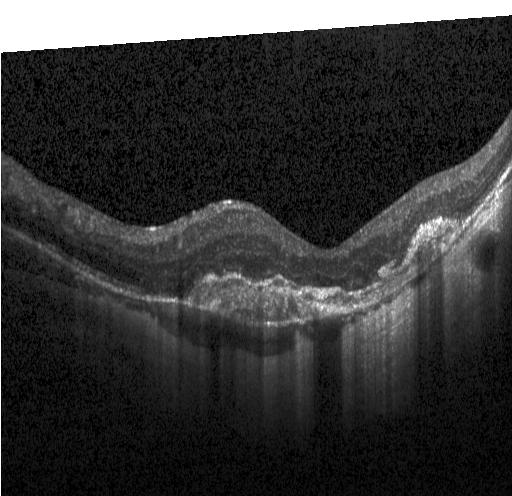
SD-OCT · Heidelberg Spectralis OCT system · retinal OCT B-scan · macular scan. Assessment: CNV.